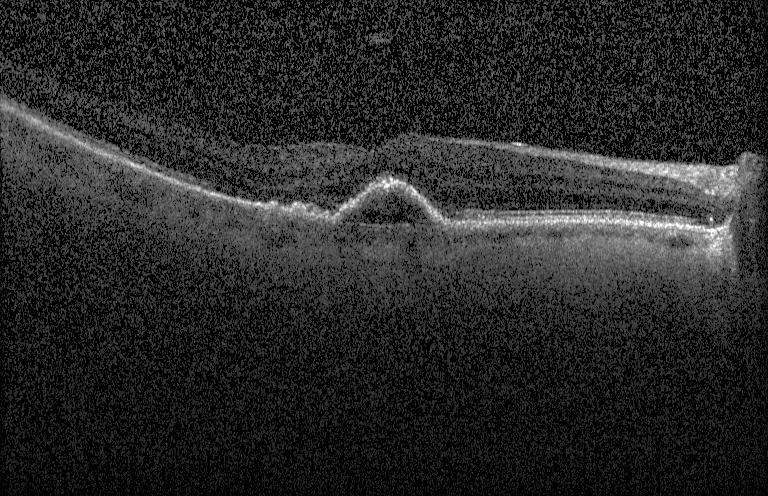 Macular OCT: choroidal neovascularization (CNV).